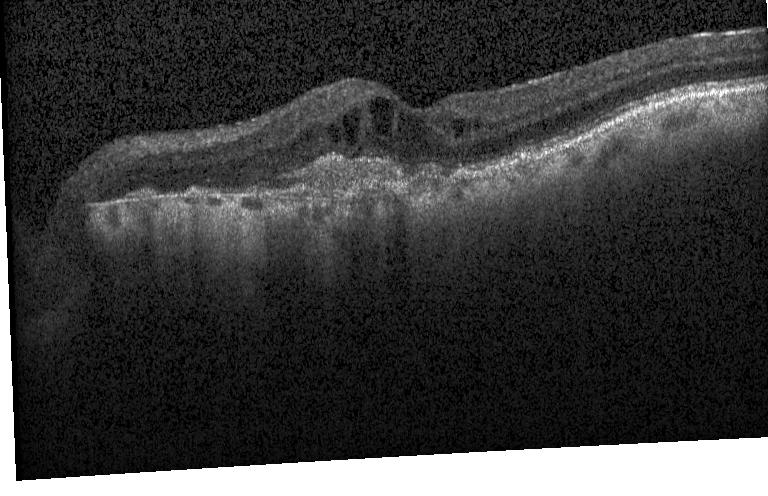 Retinal OCT cross-section. Fovea-centered. Spectral-domain OCT. Instrument: Heidelberg Spectralis. Dx: a choroidal neovascular membrane.